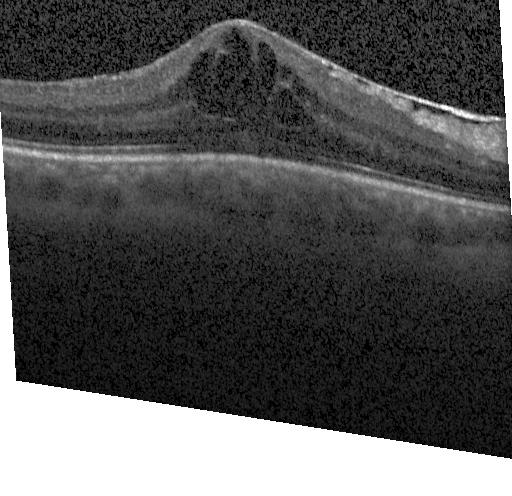

Diagnosis: DME.